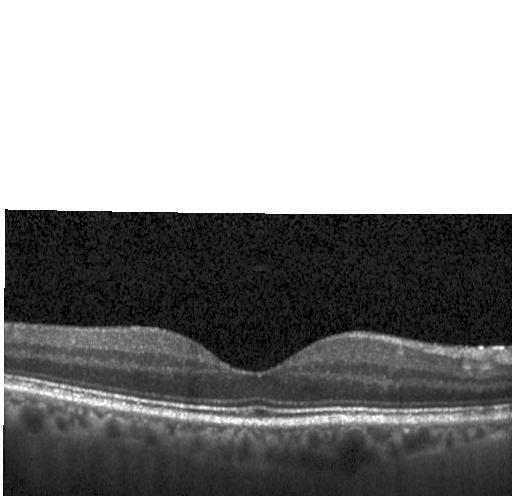
Impression: no evidence of CNV, DME, or drusen.